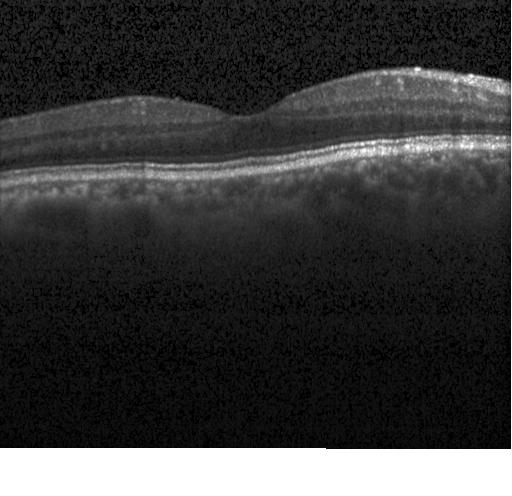

Macular OCT: no evidence of choroidal neovascularization, diabetic macular edema, or drusen.